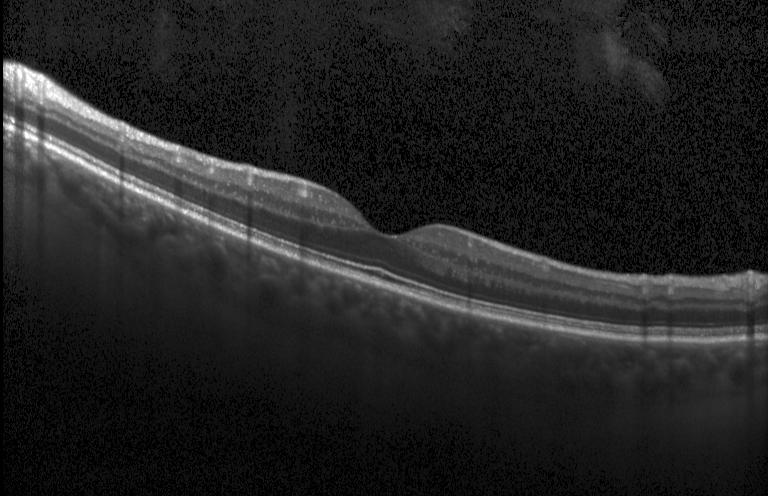 Optical coherence tomography B-scan — The scan shows no evidence of CNV, DME, or drusen.